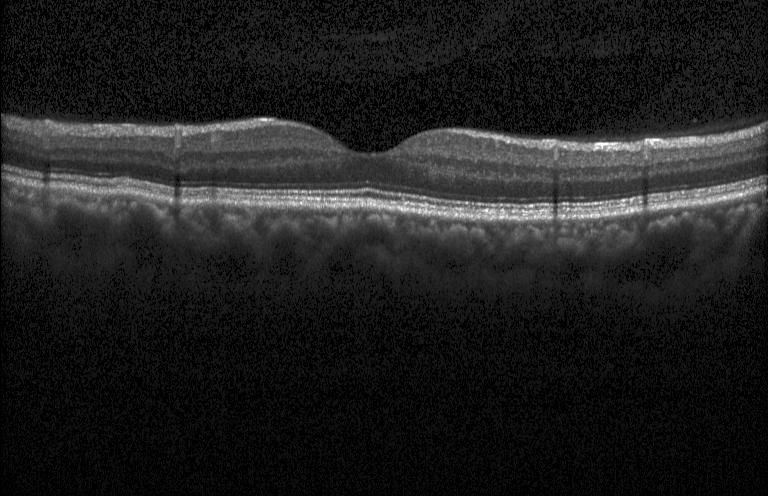 Retinal OCT cross-section. Diagnosis: no choroidal neovascularization, no diabetic macular edema, and no drusen.